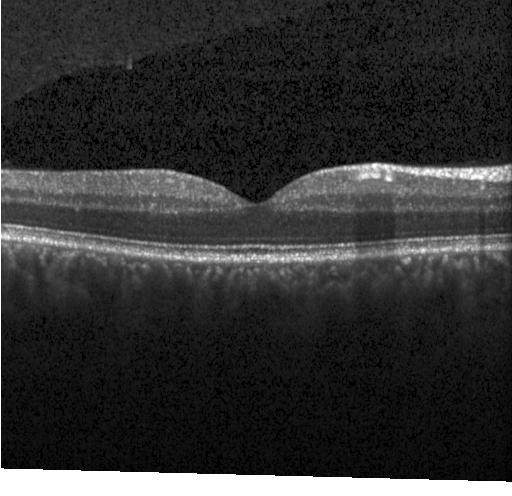

Horizontal scan through the fovea. Heidelberg Spectralis OCT system. Spectral-domain optical coherence tomography. Optical coherence tomography B-scan
Impression: no CNV, DME, or drusen.